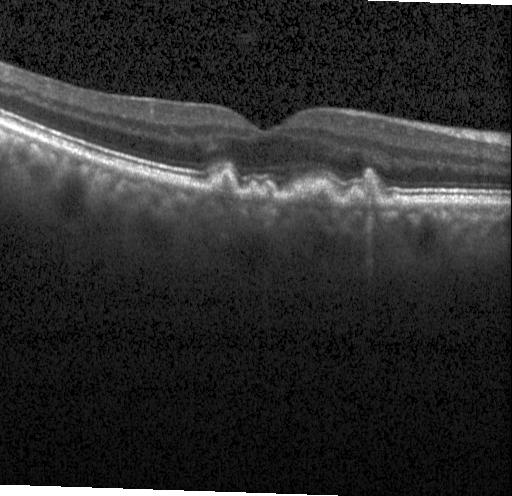
Assessment: sub-RPE drusenoid deposits.